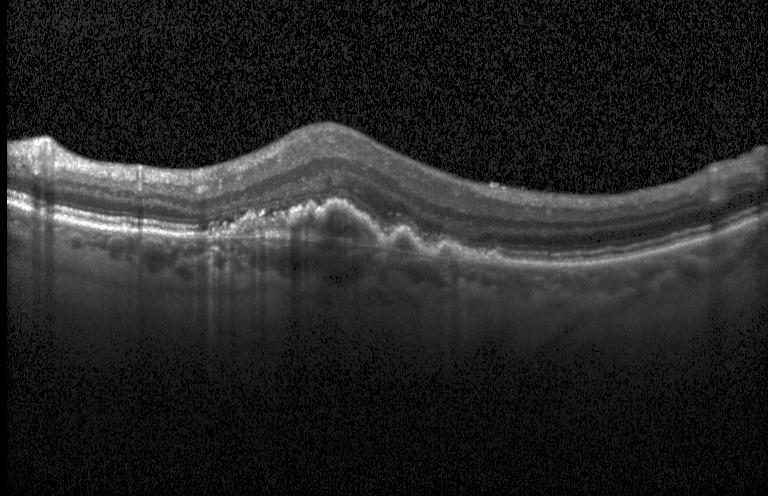

Impression: choroidal neovascularization (CNV).